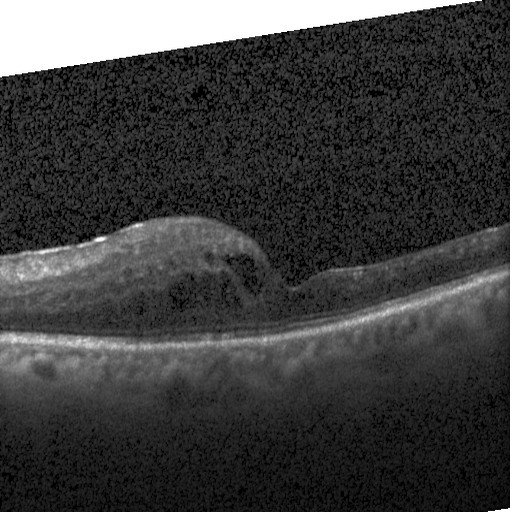
Retinal OCT cross-section
Dx: diabetic macular edema (DME).